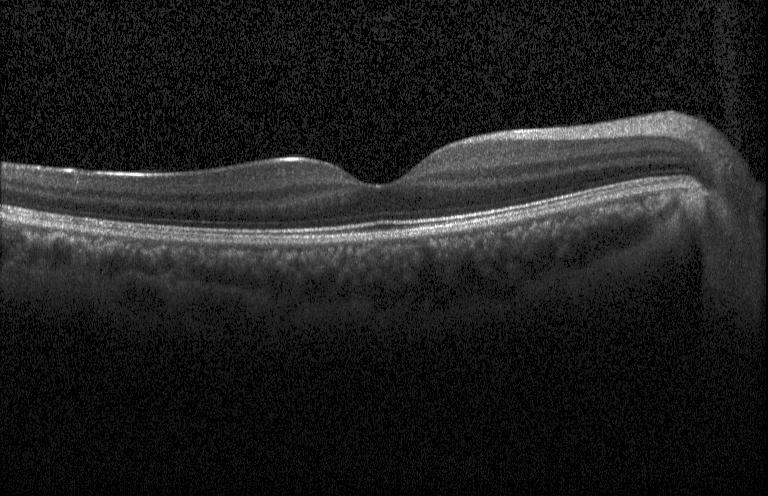

Finding: no CNV, DME, or drusen.